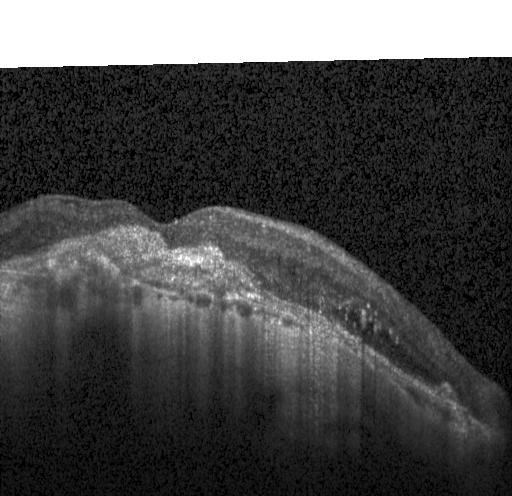
The scan shows choroidal neovascularization.